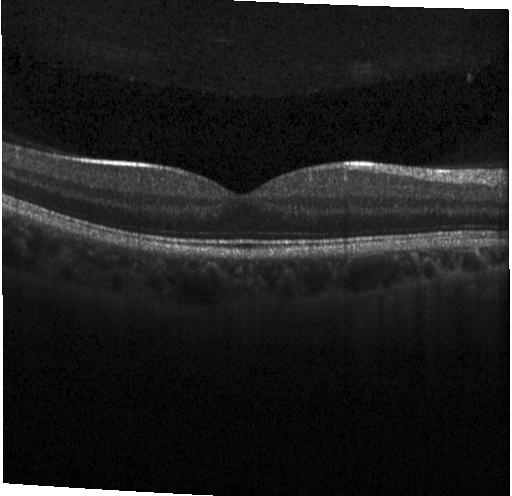
Optical coherence tomography scan. Dx: no evidence of CNV, DME, or drusen.